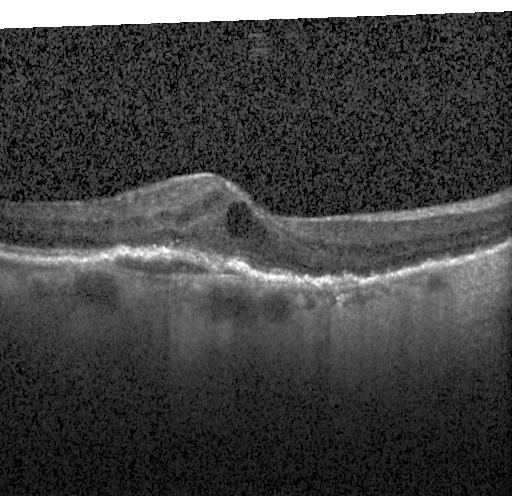 Retinal OCT cross-section — Diagnosis: choroidal neovascularization (CNV).